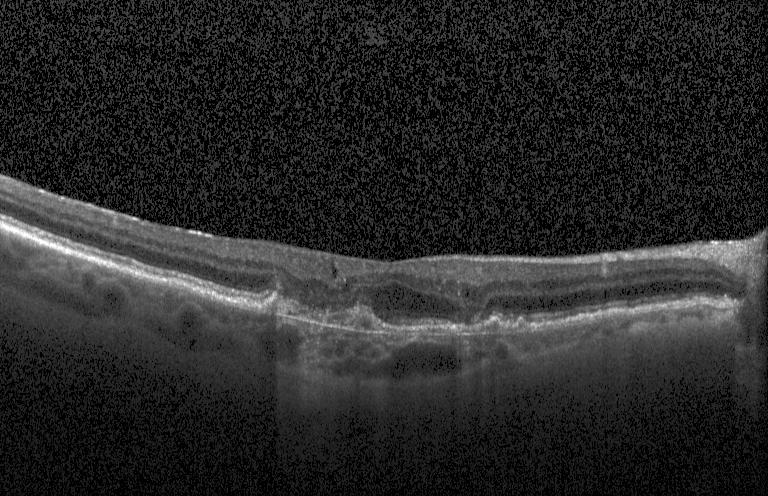 Diagnosis: choroidal neovascularization.